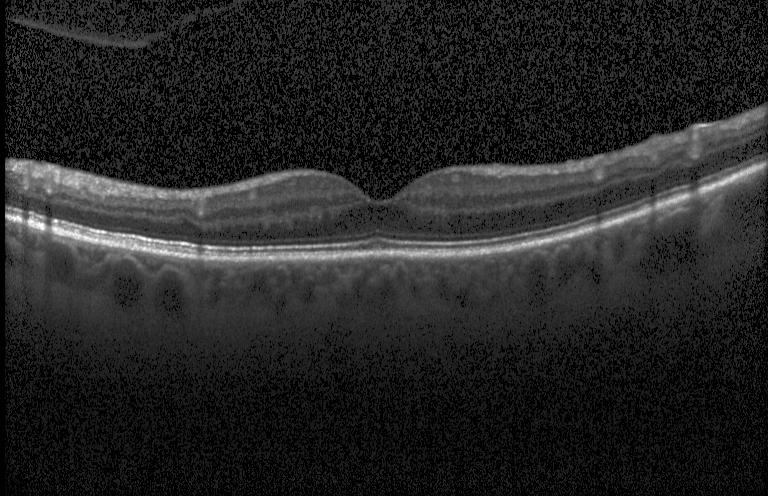
Spectral-domain optical coherence tomography; retinal OCT B-scan; Heidelberg Spectralis OCT system; fovea-centered
Assessment: no evidence of CNV, DME, or drusen.